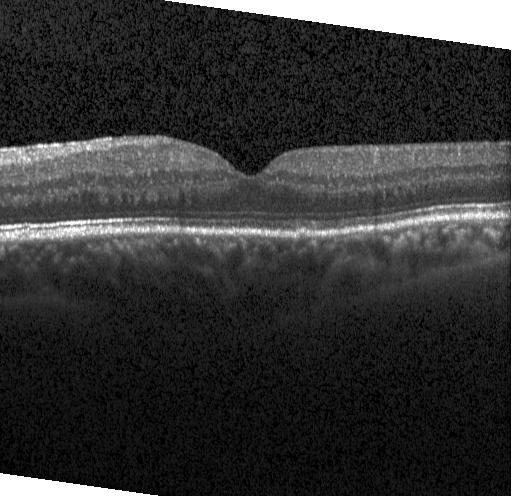

The scan shows neither CNV, DME, nor drusen.